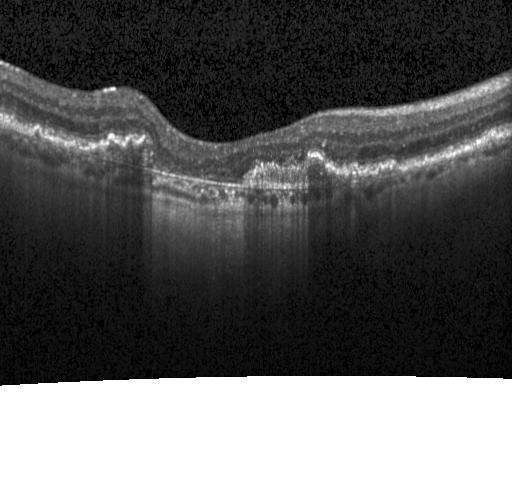
OCT B-scan. Centered on the fovea — Impression: a choroidal neovascular membrane.